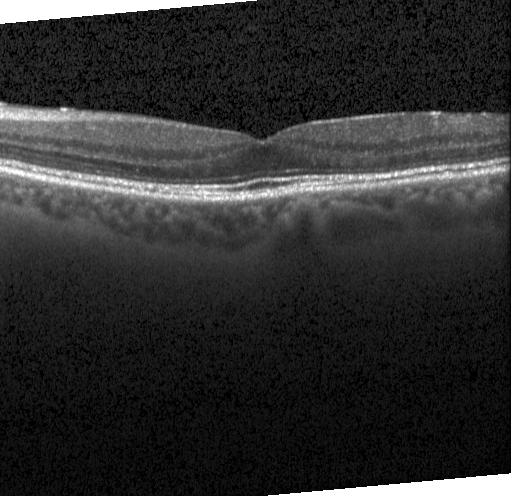 Impression: no evidence of CNV, DME, or drusen.